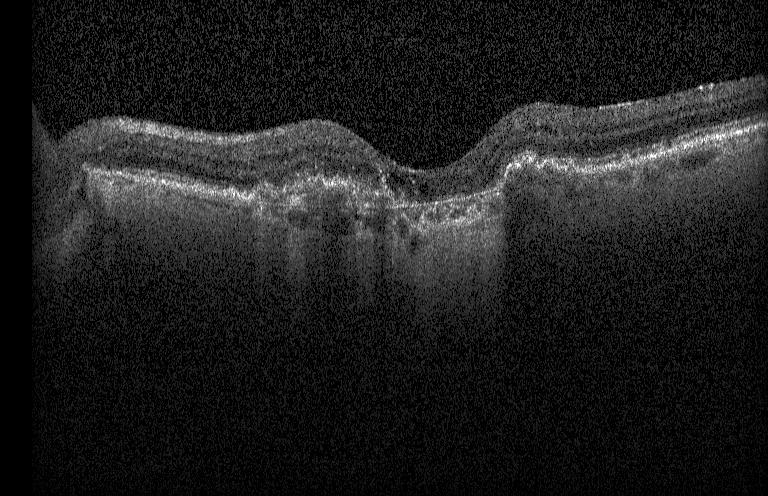
Impression: a choroidal neovascular membrane.